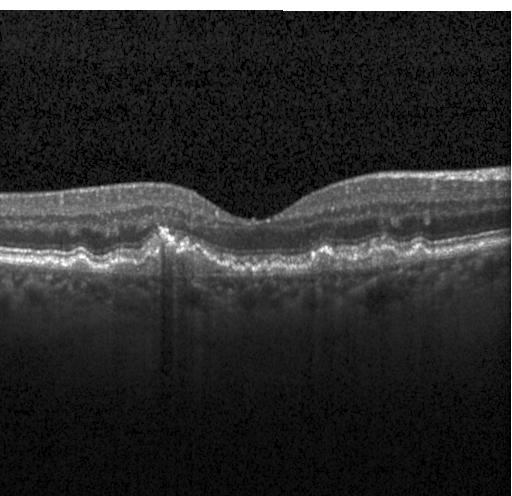
Retinal OCT cross-section. Macular scan
Finding: choroidal neovascularization.